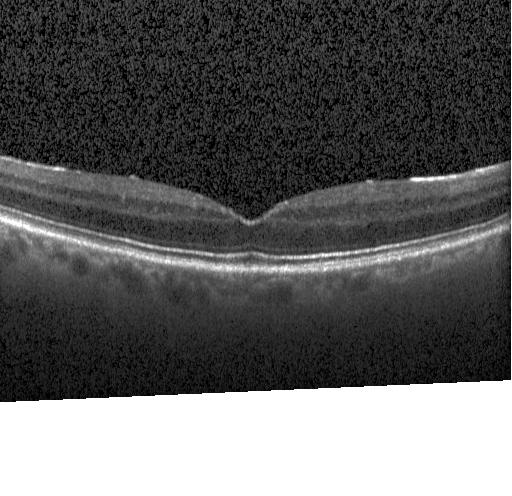

Optical coherence tomography scan — Impression: neither choroidal neovascularization, diabetic macular edema, nor drusen.